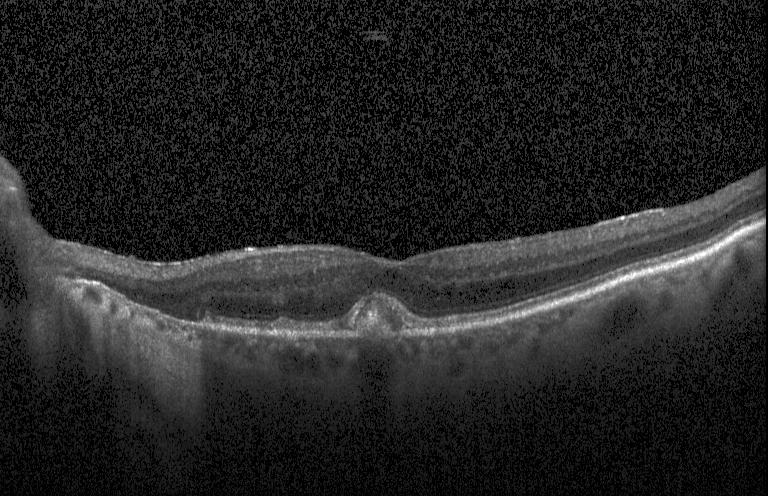
Centered on the fovea · spectral-domain optical coherence tomography · optical coherence tomography B-scan.
Finding: a choroidal neovascular membrane.